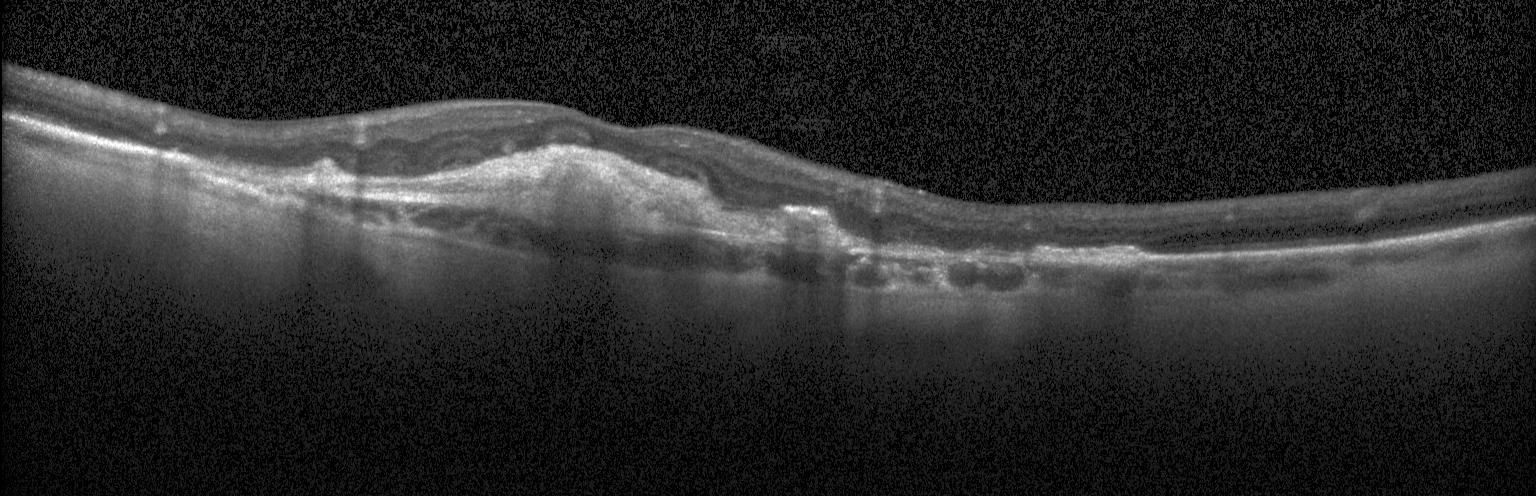
Retinal OCT cross-section; centered on the fovea; acquired on a Heidelberg Spectralis; spectral-domain OCT. A choroidal neovascular membrane.